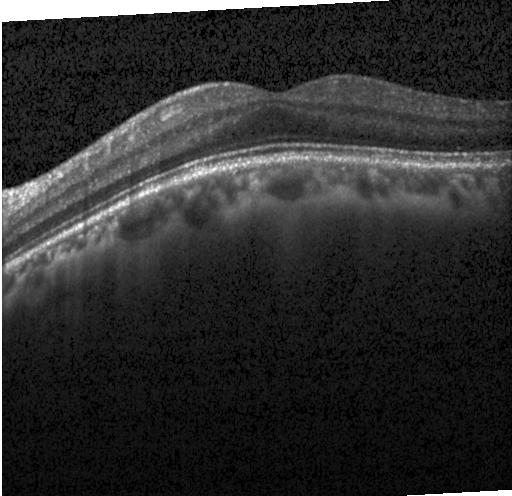

Instrument: Heidelberg Spectralis, optical coherence tomography B-scan — The scan shows no CNV, no DME, and no drusen.